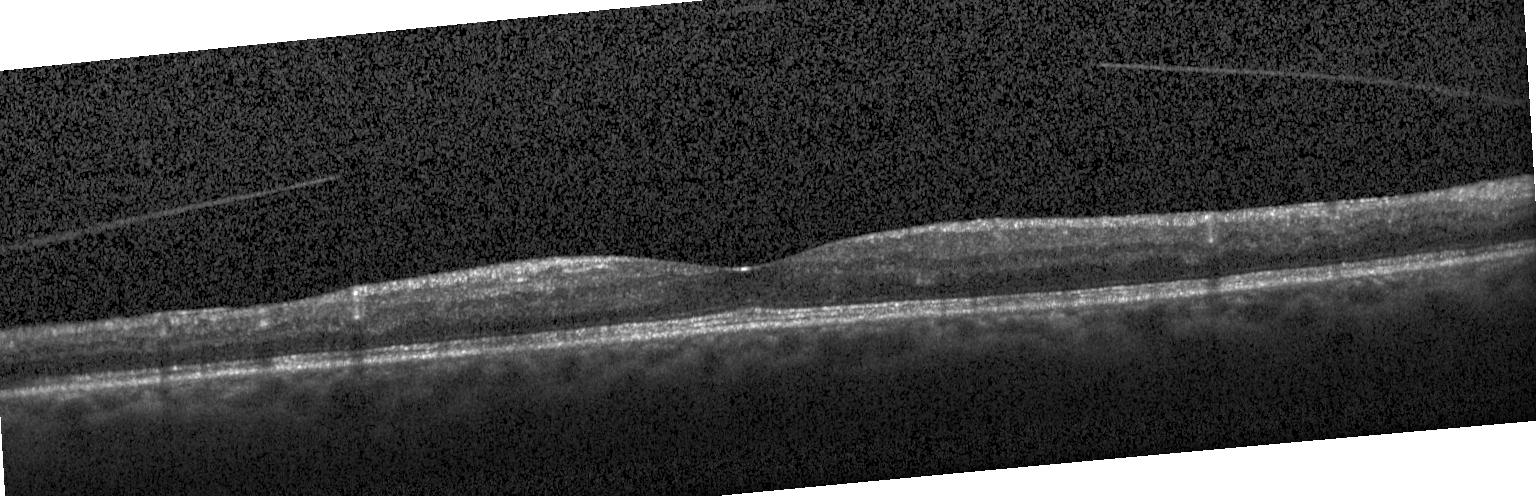
Optical coherence tomography scan.
Impression: DME.